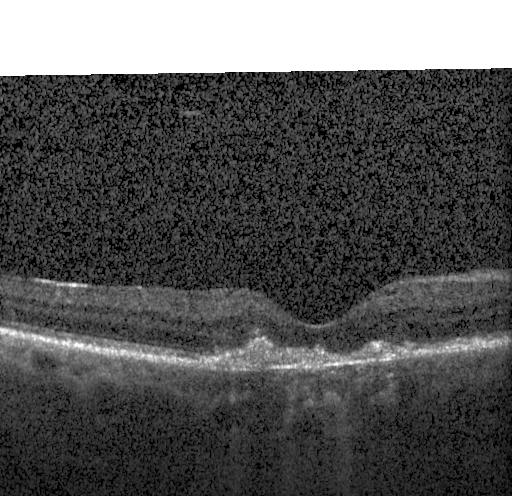

OCT B-scan. Assessment: a choroidal neovascular membrane.